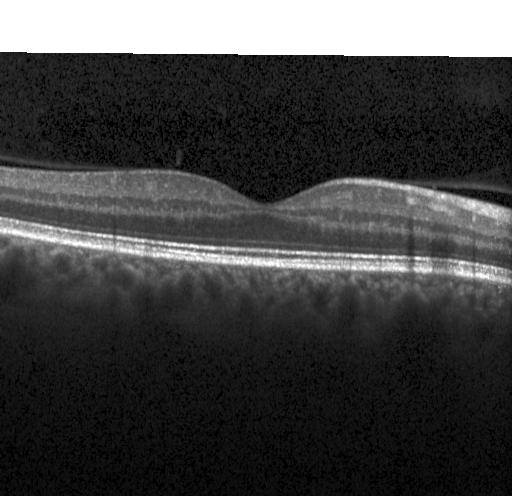
Macular scan. OCT B-scan
Dx: neither CNV, DME, nor drusen.